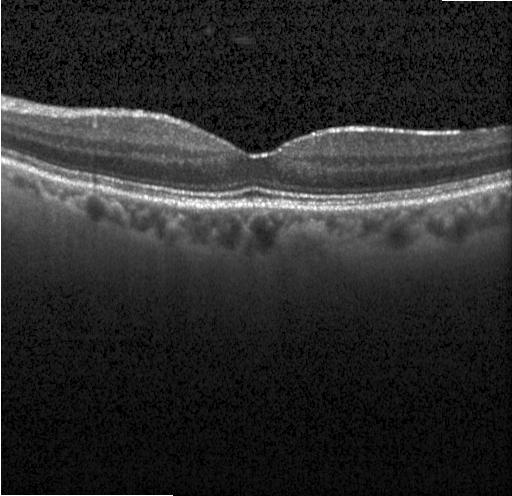
Through the macula · acquired on a Heidelberg Spectralis · retinal OCT B-scan.
Diagnosis: no choroidal neovascularization, no diabetic macular edema, and no drusen.